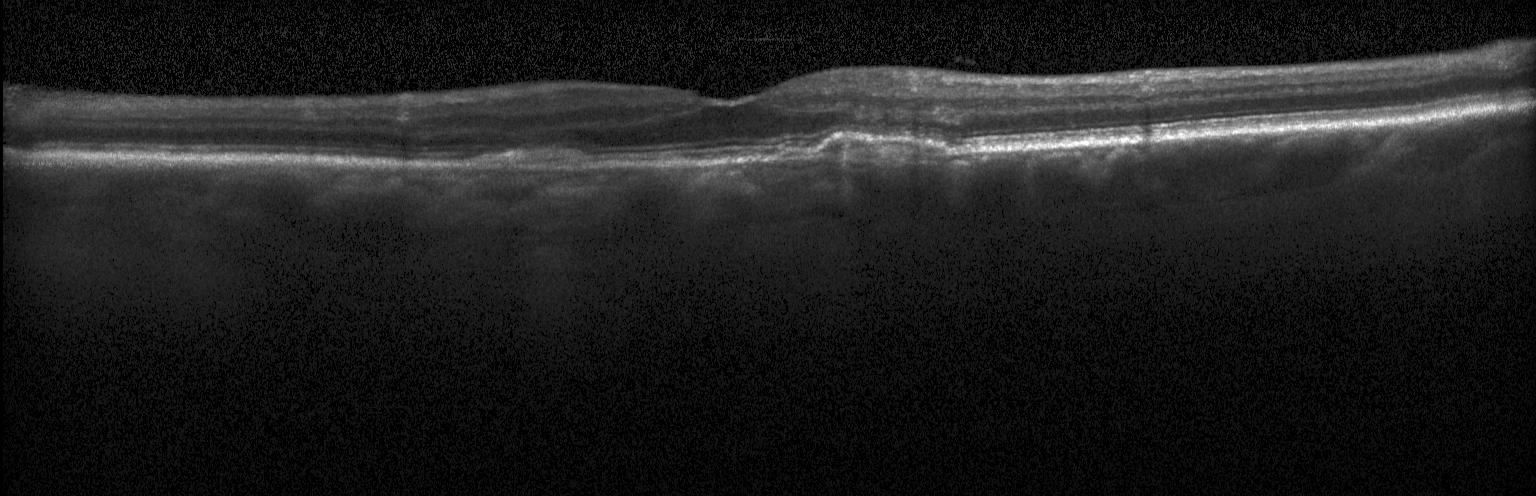

Heidelberg Spectralis OCT system. Retinal OCT B-scan. SD-OCT
This B-scan demonstrates a choroidal neovascular membrane.